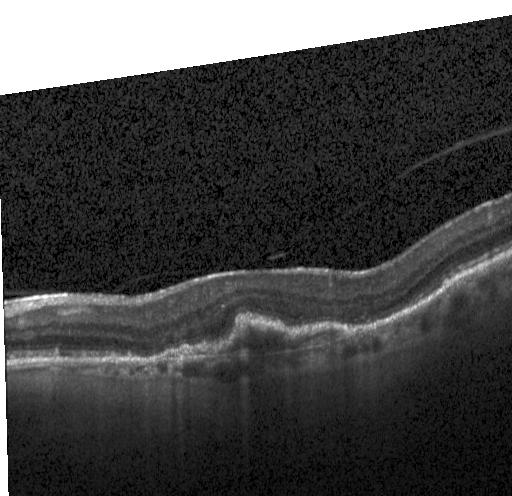

A choroidal neovascular membrane.